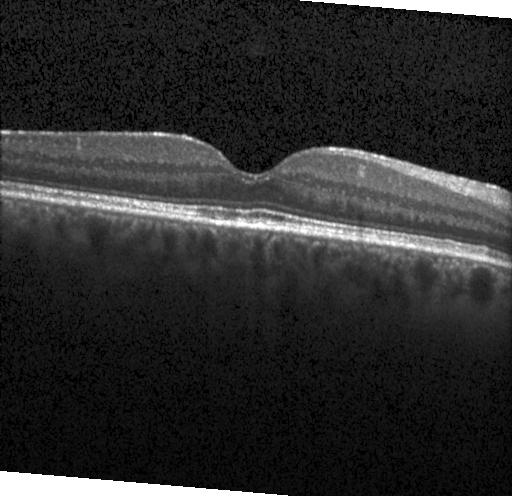

Retinal OCT cross-section; spectral-domain optical coherence tomography
Finding: no choroidal neovascularization, no diabetic macular edema, and no drusen.